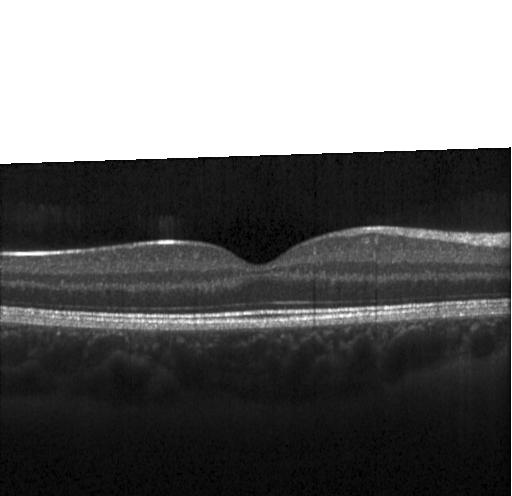 Optical coherence tomography scan.
The scan shows neither CNV, DME, nor drusen.